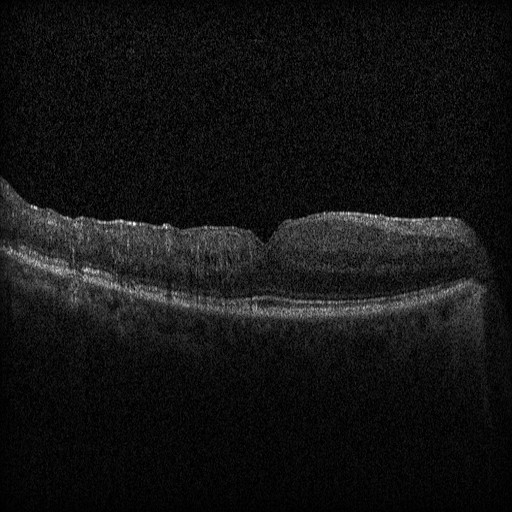
Acquired on a Heidelberg Spectralis · retinal OCT cross-section · fovea-centered — This B-scan demonstrates diabetic macular edema (DME).